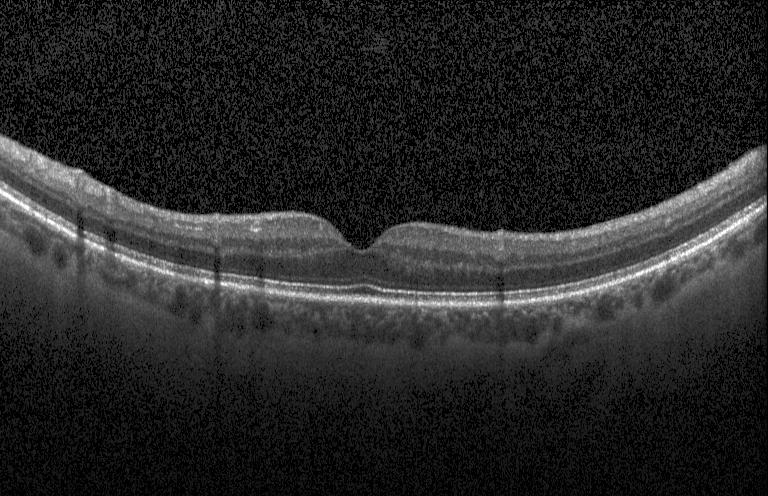

Heidelberg Spectralis, OCT line scan, SD-OCT, macular scan. Impression: no choroidal neovascularization, diabetic macular edema, or drusen.